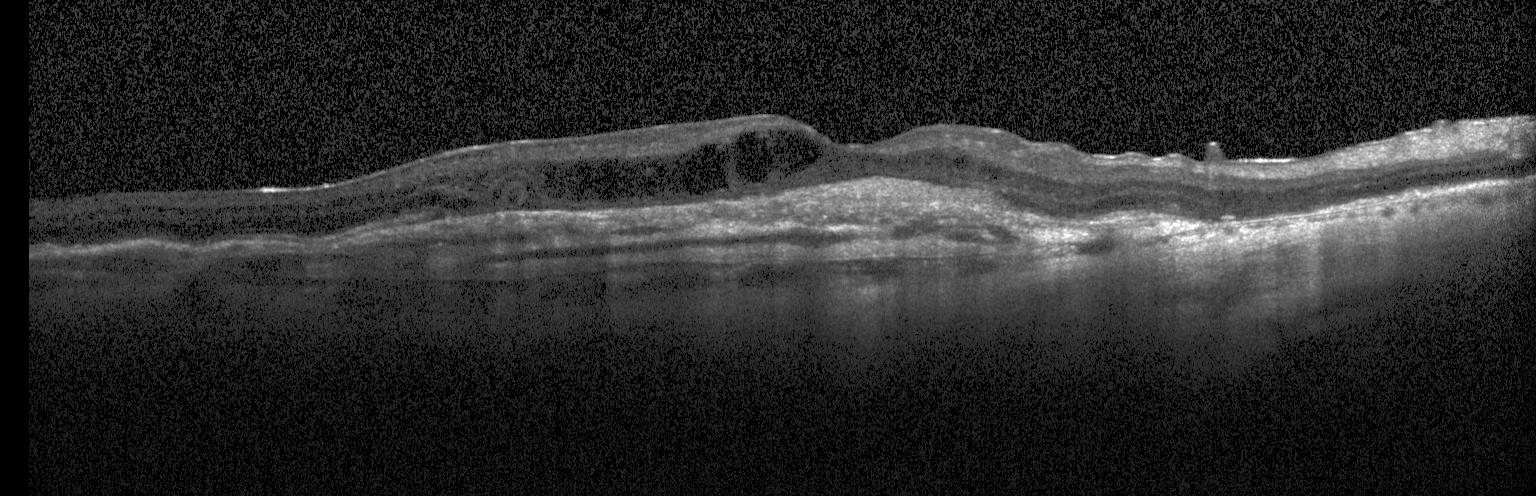
OCT B-scan
Dx: a choroidal neovascular membrane.